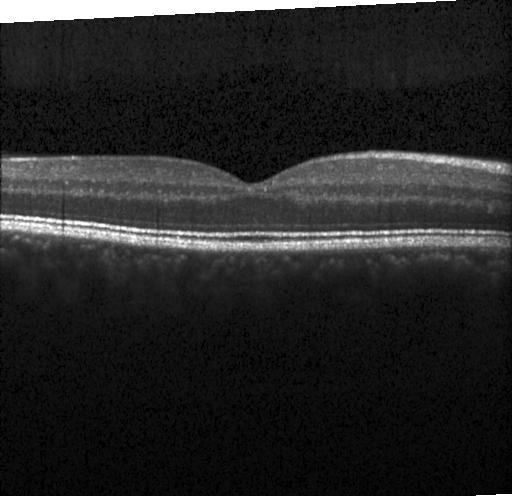

The scan shows no CNV, no DME, and no drusen.